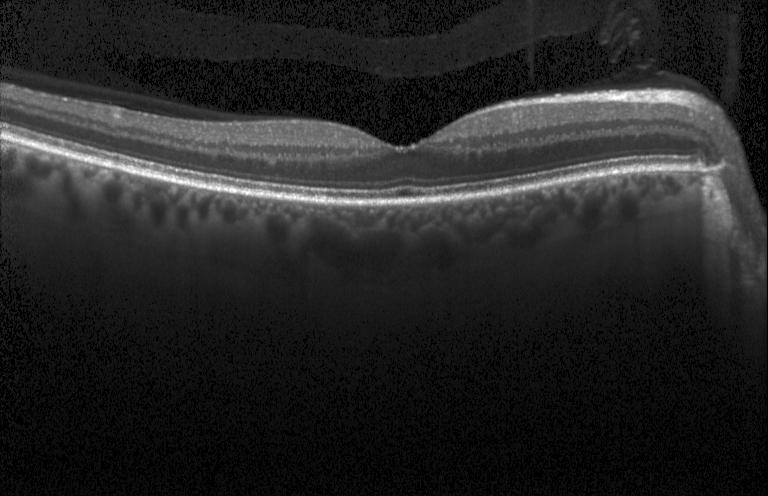 OCT B-scan showing no CNV, no DME, and no drusen.